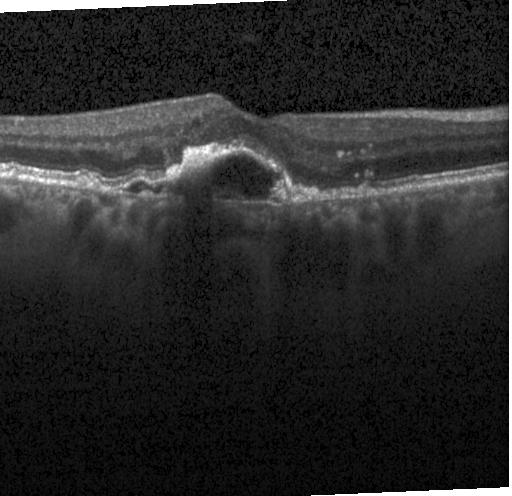

OCT line scan. This B-scan demonstrates CNV.